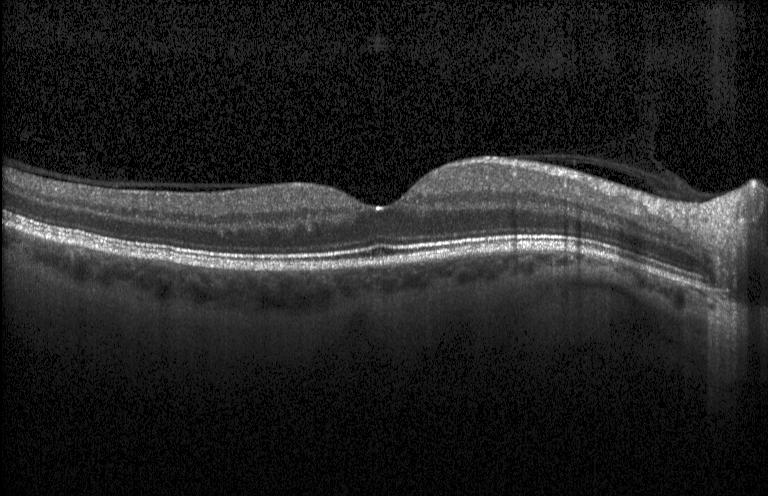 Horizontal scan through the fovea, retinal OCT cross-section, spectral-domain optical coherence tomography
No choroidal neovascularization, diabetic macular edema, or drusen.